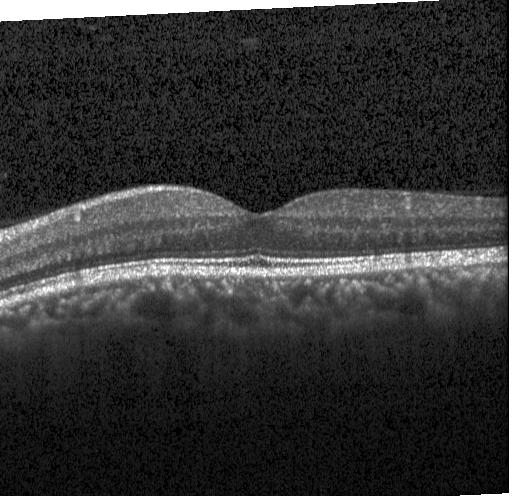

Optical coherence tomography scan, macular scan, SD-OCT — Impression: no choroidal neovascularization, diabetic macular edema, or drusen.